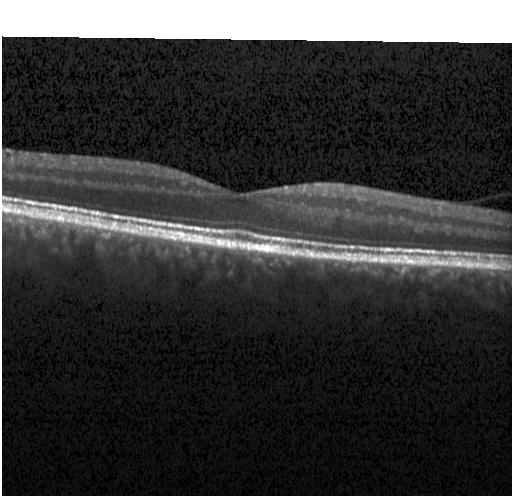
Instrument: Heidelberg Spectralis · through the macula · OCT B-scan · SD-OCT. Finding: no evidence of choroidal neovascularization, diabetic macular edema, or drusen.